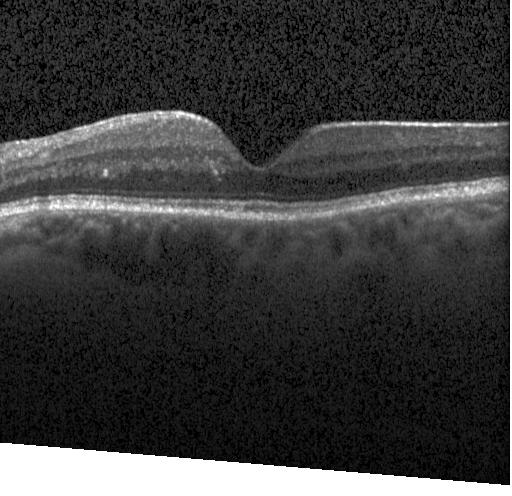 Macular scan · Heidelberg Spectralis · SD-OCT · optical coherence tomography scan.
The scan shows no CNV, no DME, and no drusen.